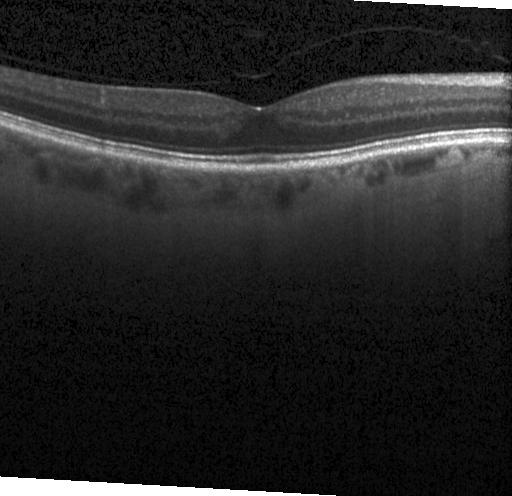

Through the macula · retinal OCT B-scan — Finding: no evidence of choroidal neovascularization, diabetic macular edema, or drusen.